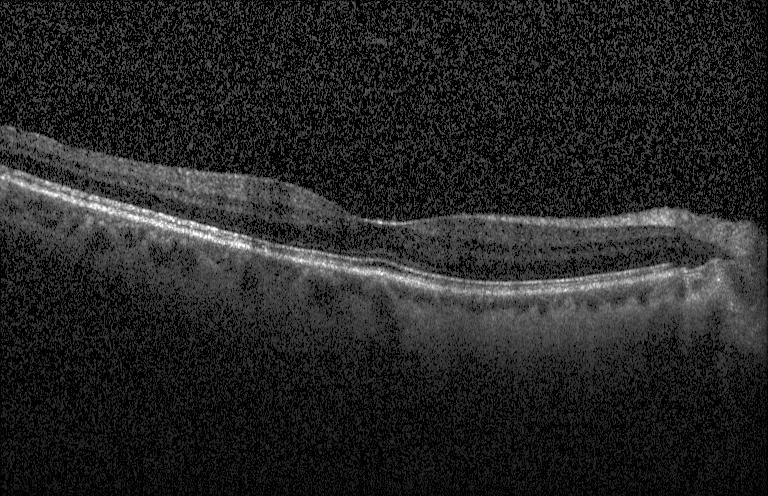 The scan shows neither choroidal neovascularization, diabetic macular edema, nor drusen.